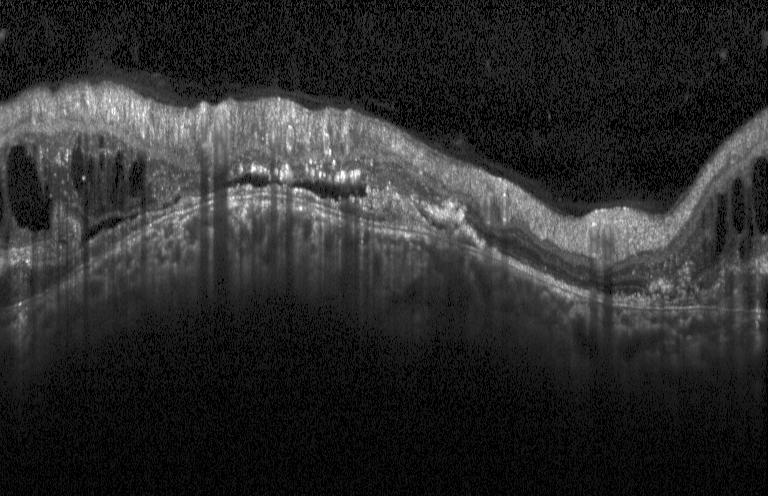
Optical coherence tomography scan · spectral-domain optical coherence tomography. OCT finding: choroidal neovascularization.